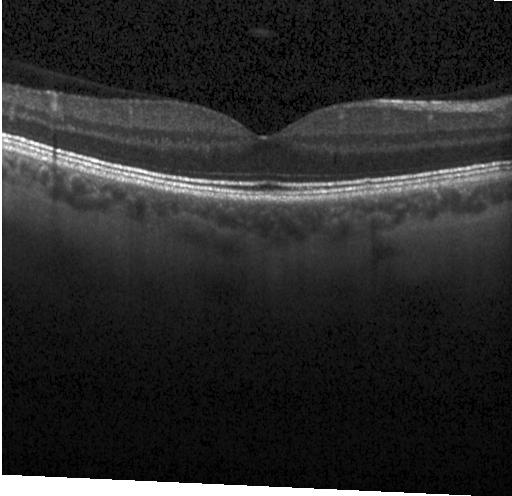

Retinal OCT cross-section, fovea-centered. The scan shows no choroidal neovascularization, diabetic macular edema, or drusen.